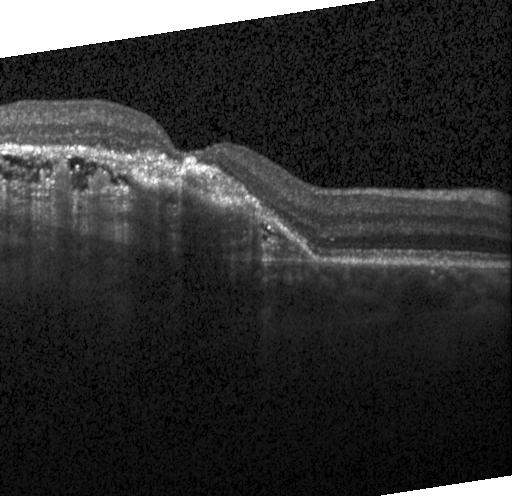 Centered on the fovea · OCT B-scan.
The scan shows a choroidal neovascular membrane.